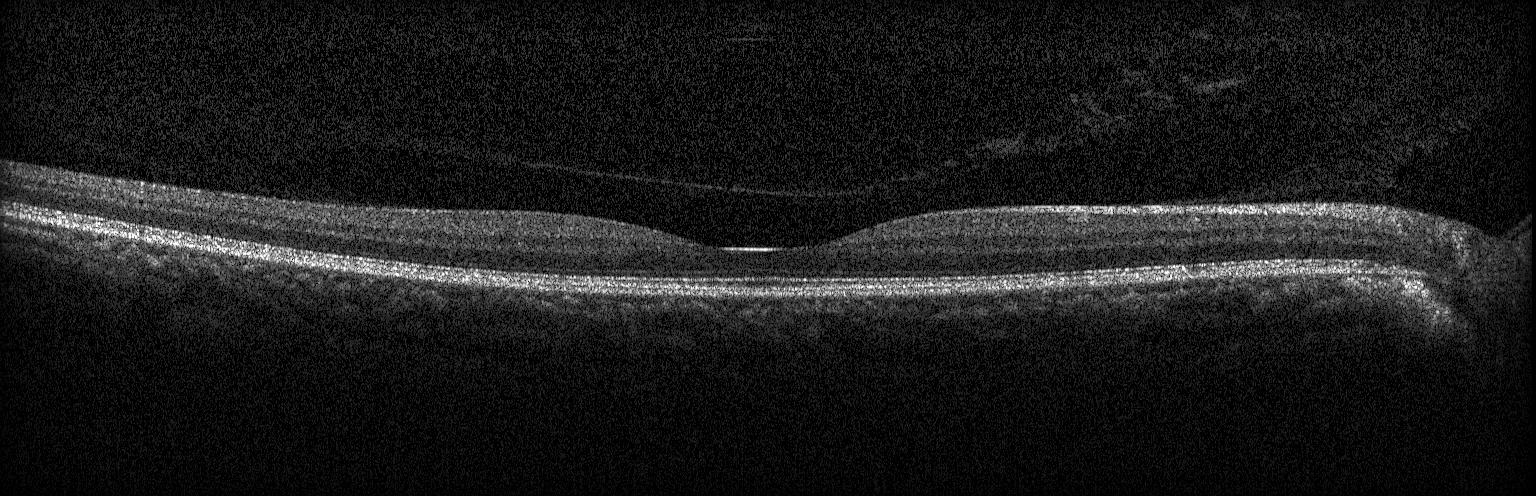

Diagnosis: no CNV, DME, or drusen.